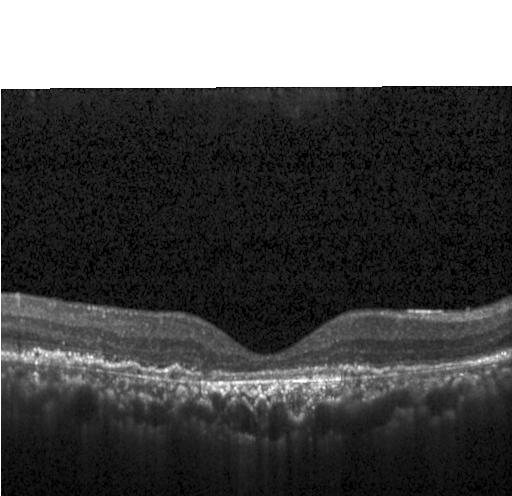

A choroidal neovascular membrane.